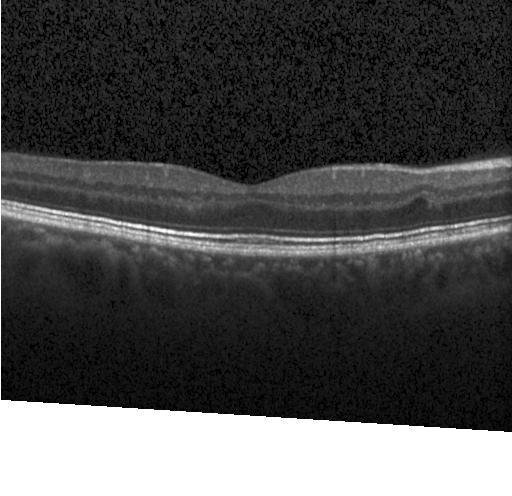

Retinal OCT cross-section; macular scan; Heidelberg Spectralis OCT system
This B-scan demonstrates no evidence of choroidal neovascularization, diabetic macular edema, or drusen.